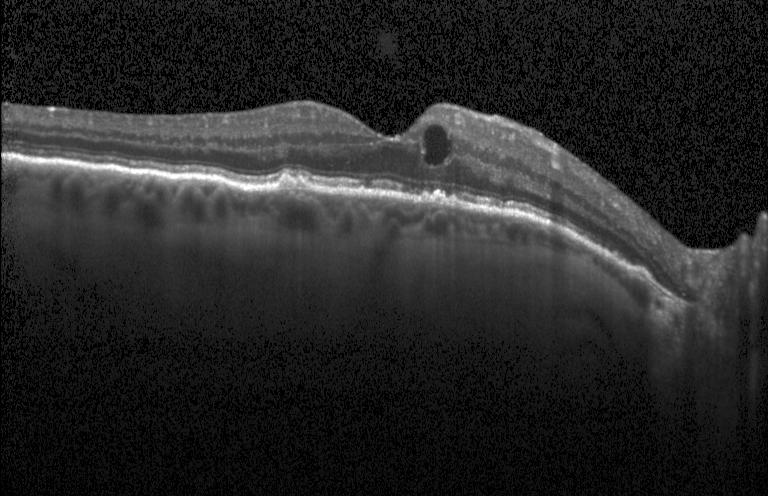 Finding: a choroidal neovascular membrane.